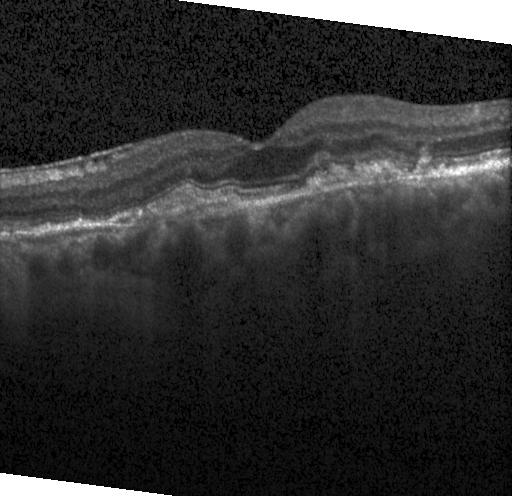
OCT B-scan showing choroidal neovascularization (CNV).